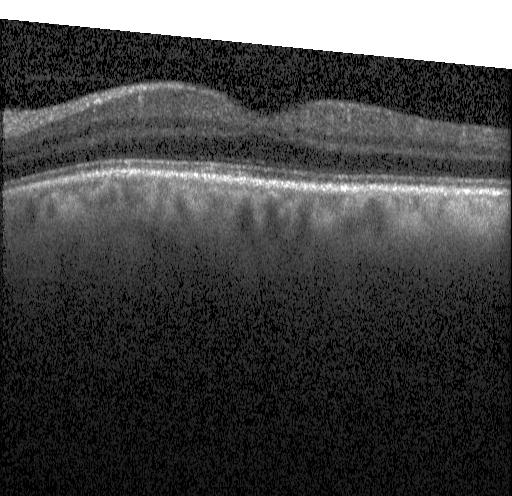
OCT B-scan.
OCT finding: neither choroidal neovascularization, diabetic macular edema, nor drusen.